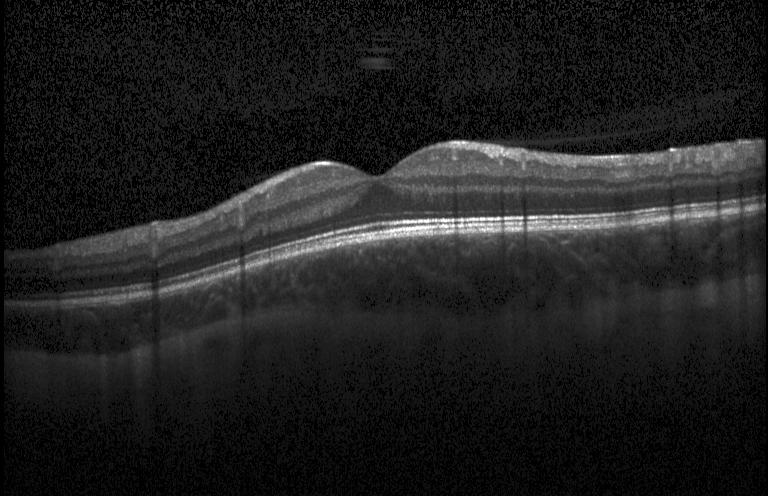 Horizontal scan through the fovea, optical coherence tomography B-scan.
Impression: no evidence of CNV, DME, or drusen.